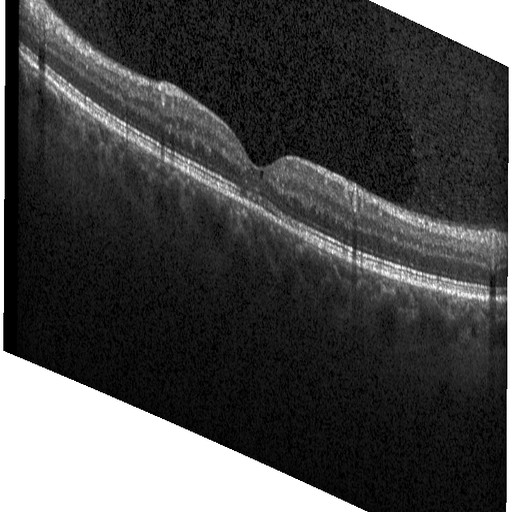

Assessment: diabetic macular edema.